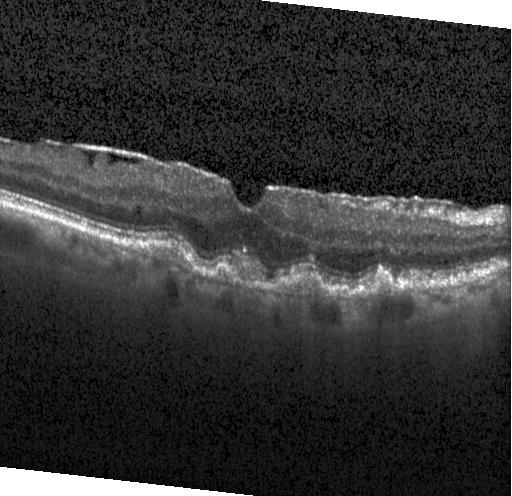 Through the macula. Optical coherence tomography B-scan. Heidelberg Spectralis. Spectral-domain optical coherence tomography
Diagnosis: sub-RPE drusenoid deposits.